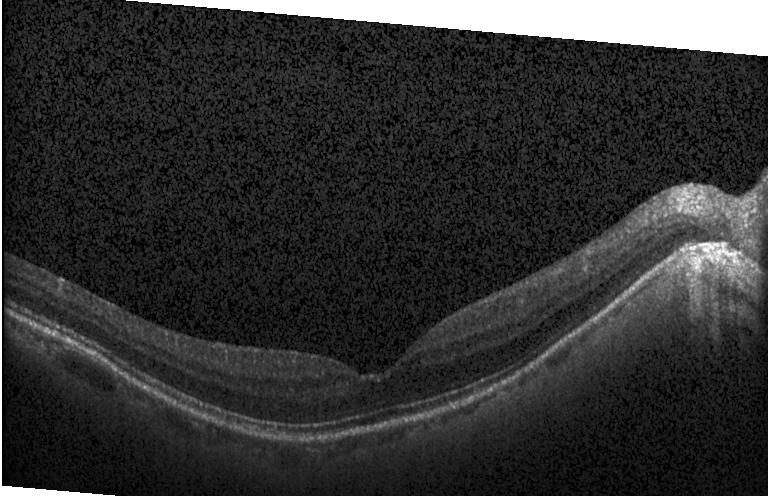 Through the macula. OCT line scan
Diagnosis: no choroidal neovascularization, diabetic macular edema, or drusen.